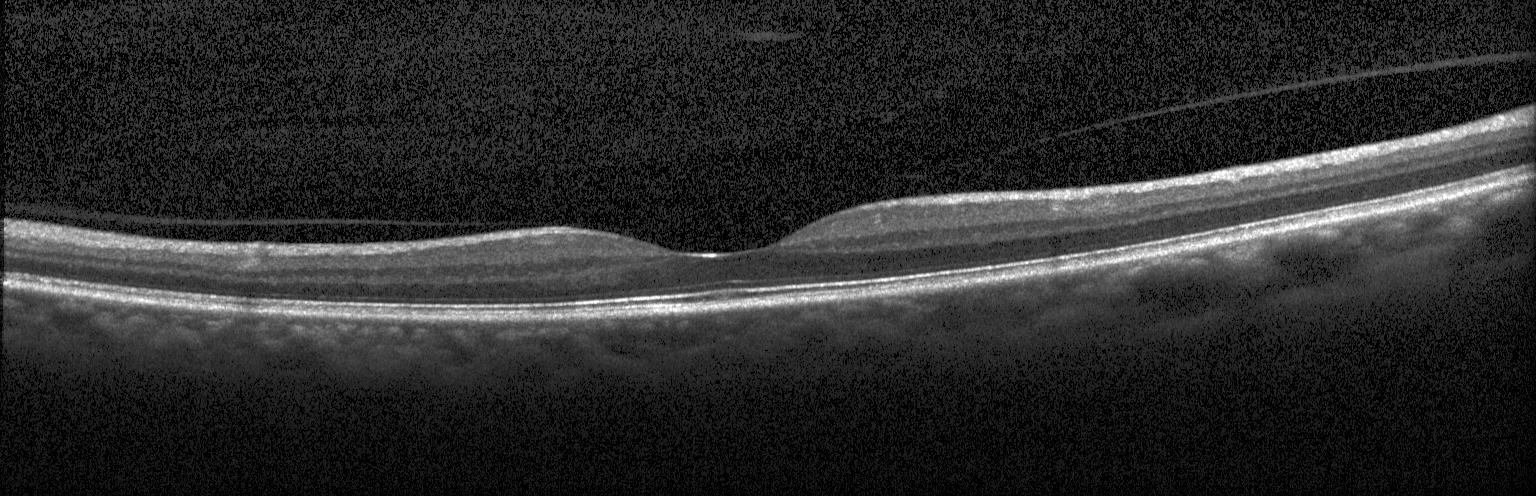
Macular scan, OCT line scan
Finding: no CNV, DME, or drusen.